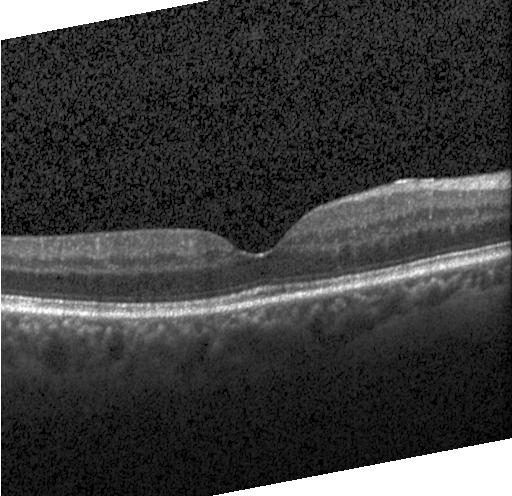

Finding: no choroidal neovascularization, diabetic macular edema, or drusen.